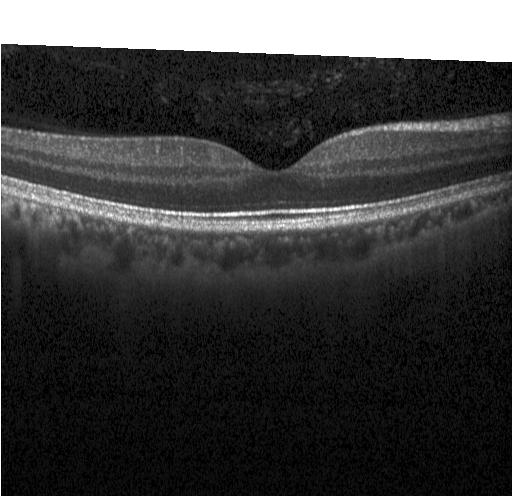 Diagnosis: no evidence of choroidal neovascularization, diabetic macular edema, or drusen.